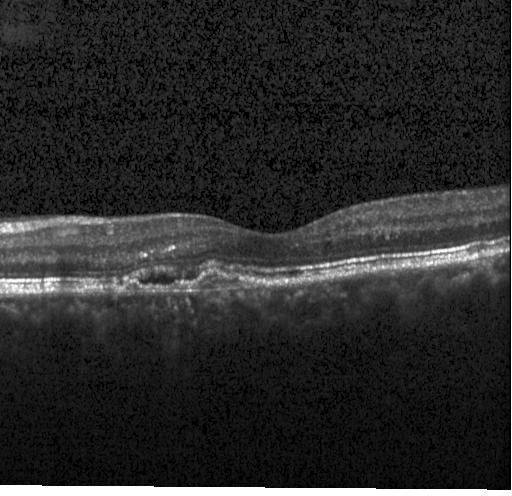 Through the macula, retinal OCT B-scan
Assessment: a choroidal neovascular membrane.